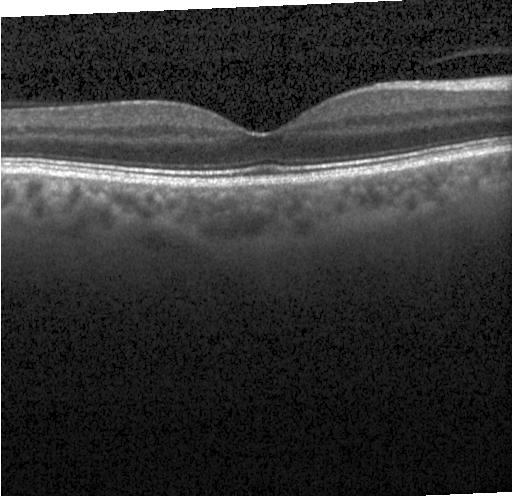

Retinal OCT B-scan, Heidelberg Spectralis OCT system, spectral-domain OCT — Finding: no CNV, DME, or drusen.